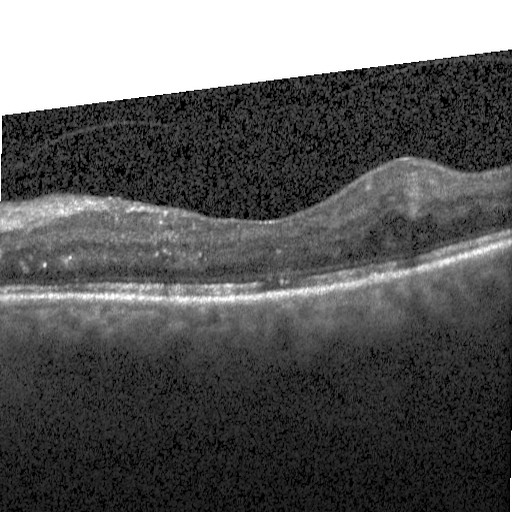 Centered on the fovea · retinal OCT cross-section · acquired on a Heidelberg Spectralis. Finding: diabetic macular edema (DME).